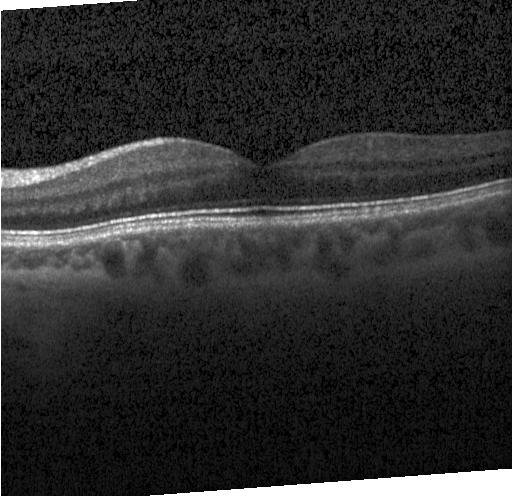 Optical coherence tomography B-scan, fovea-centered, spectral-domain optical coherence tomography. Macular OCT: no CNV, DME, or drusen.